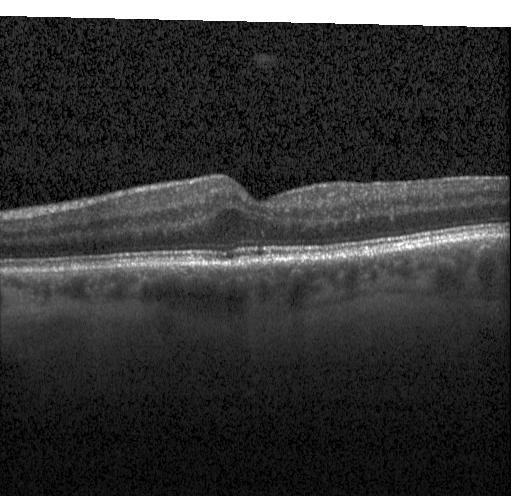
Assessment: diabetic macular edema (DME).